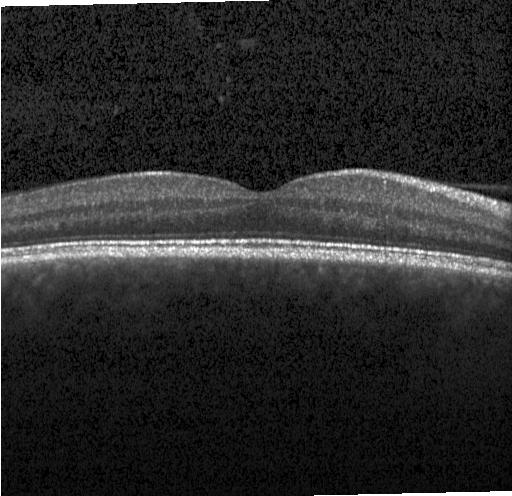
OCT B-scan.
The scan shows no choroidal neovascularization, no diabetic macular edema, and no drusen.